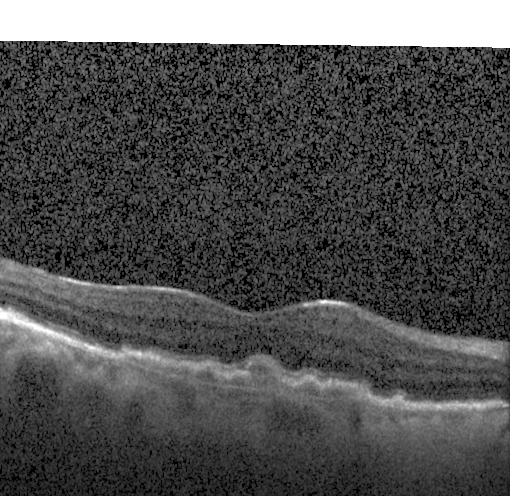
Spectral-domain optical coherence tomography; retinal OCT cross-section; Heidelberg Spectralis OCT system — Impression: a choroidal neovascular membrane.